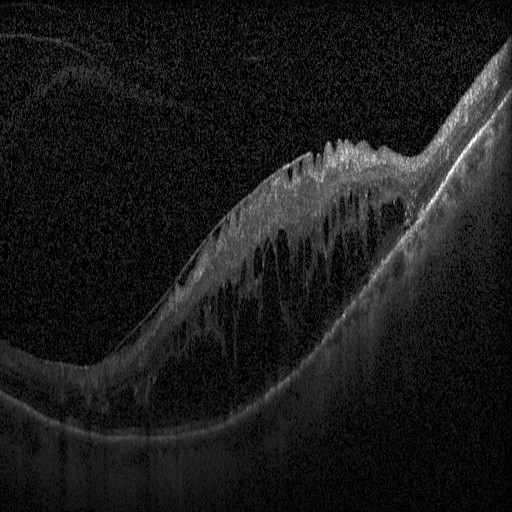 Macular OCT: diabetic macular edema (DME).